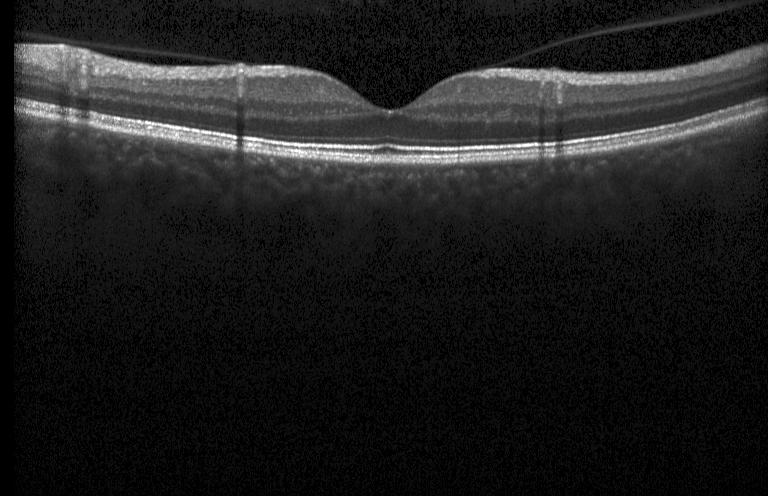 No evidence of choroidal neovascularization, diabetic macular edema, or drusen.